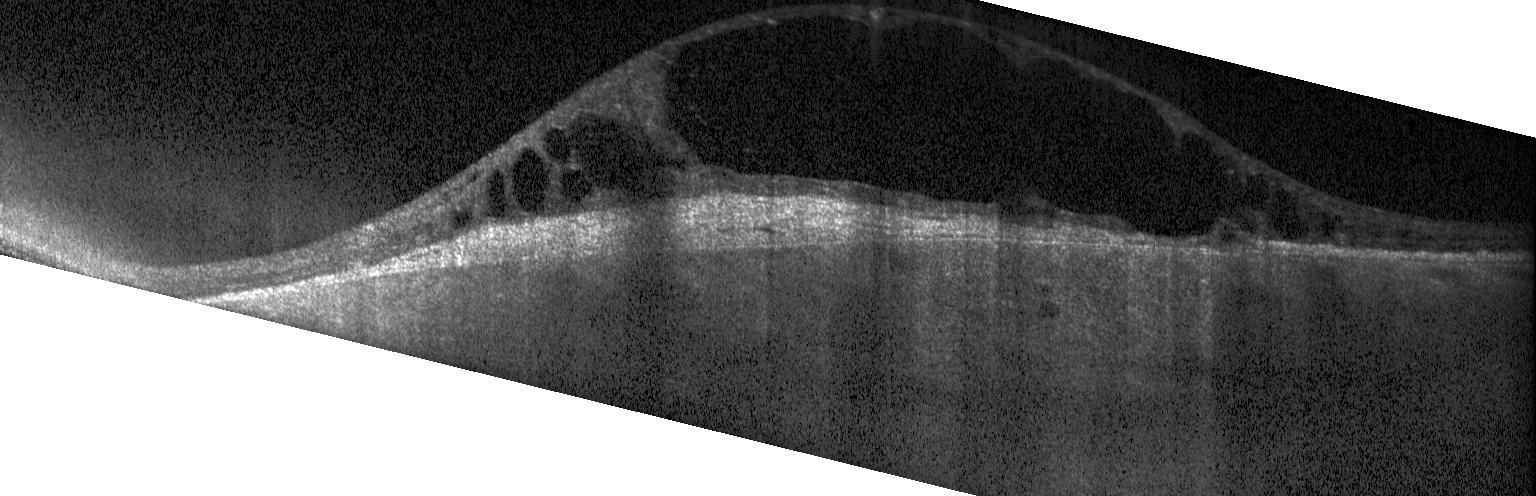

Optical coherence tomography scan; Heidelberg Spectralis; spectral-domain optical coherence tomography.
Finding: choroidal neovascularization (CNV).